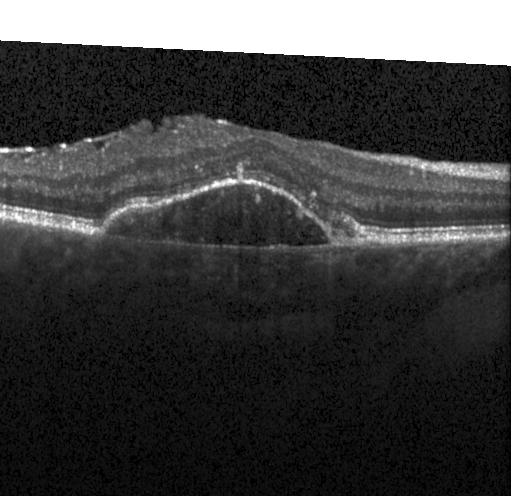
Optical coherence tomography B-scan.
Macular OCT: choroidal neovascularization.